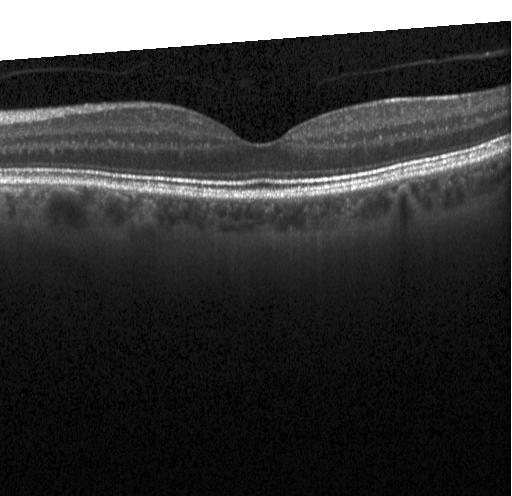 Retinal OCT B-scan — Impression: neither CNV, DME, nor drusen.